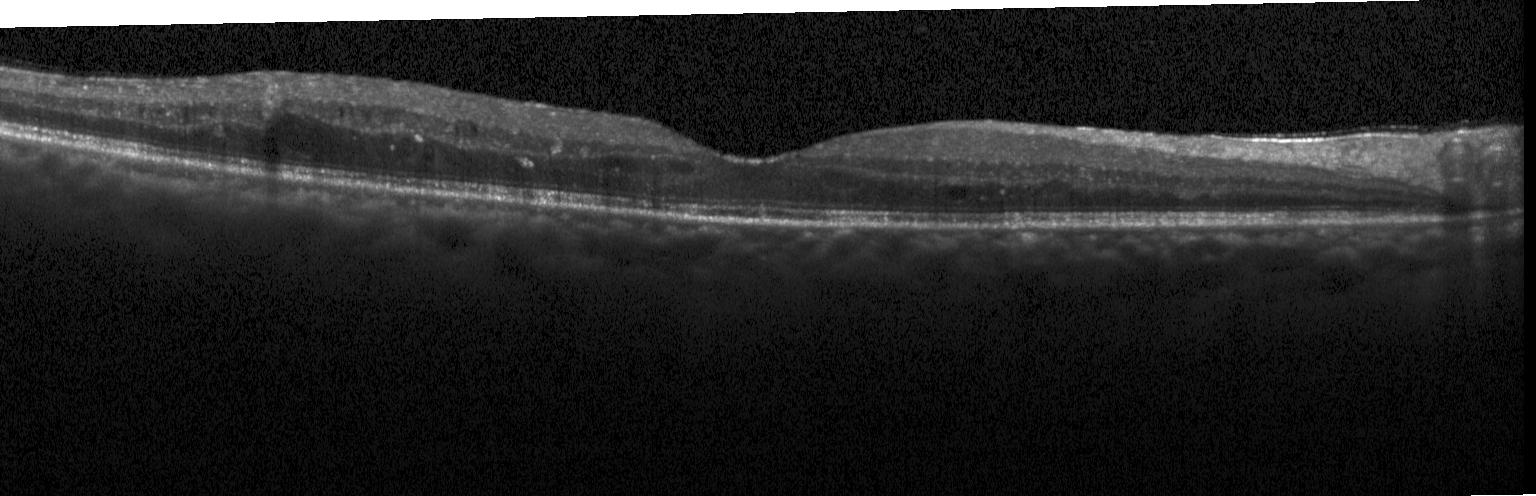

Heidelberg Spectralis; OCT line scan; SD-OCT; fovea-centered. Diagnosis: diabetic macular edema.